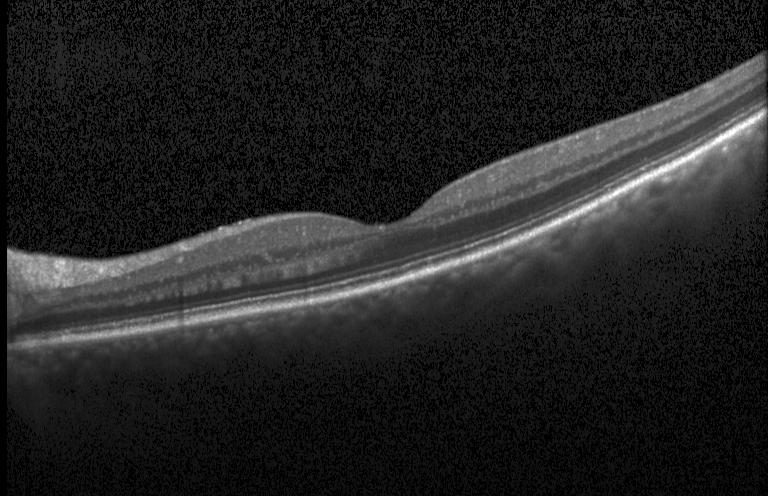 Assessment: neither CNV, DME, nor drusen.